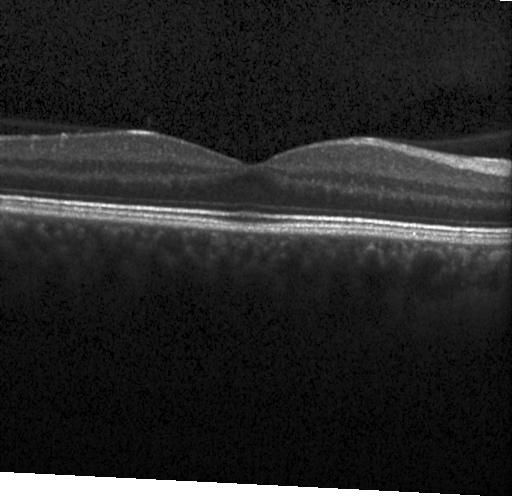 OCT line scan. SD-OCT. Horizontal scan through the fovea. Heidelberg Spectralis. Diagnosis: neither CNV, DME, nor drusen.